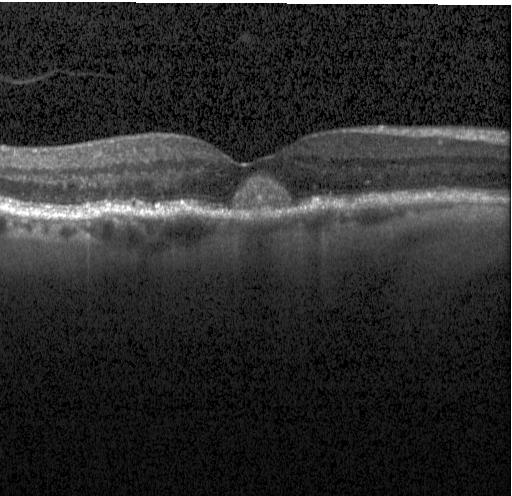 OCT finding: sub-RPE drusenoid deposits.